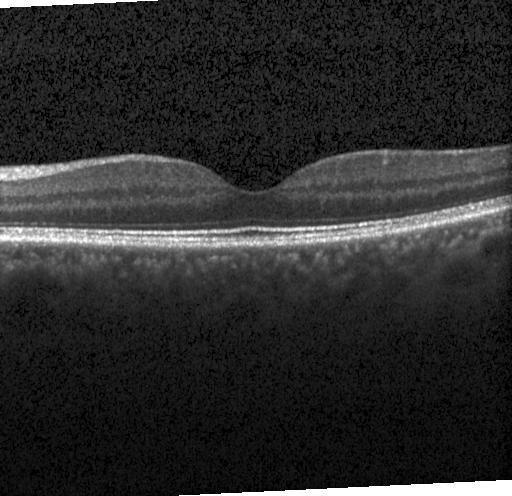 OCT line scan · fovea-centered · Heidelberg Spectralis
Diagnosis: no choroidal neovascularization, no diabetic macular edema, and no drusen.